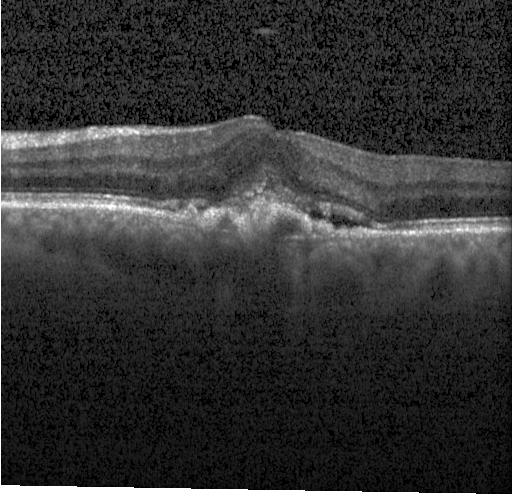

CNV.